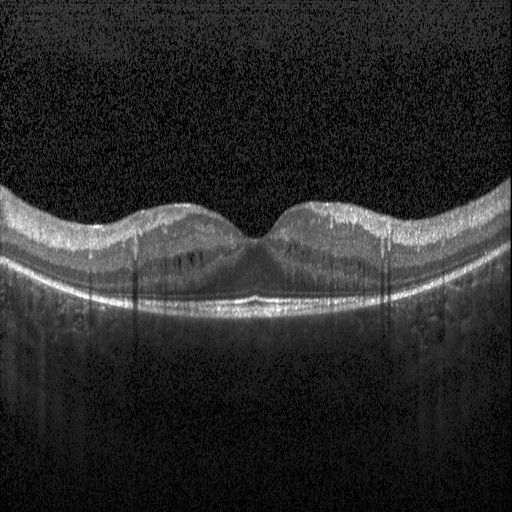
OCT scan showing DME.